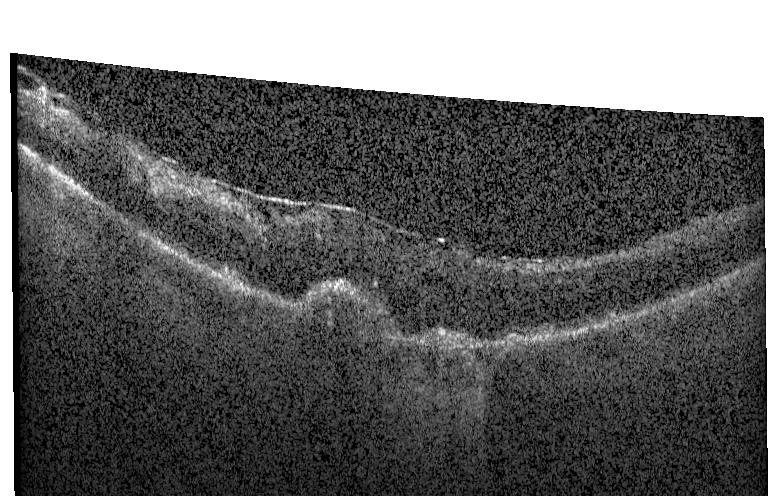
OCT B-scan showing choroidal neovascularization (CNV).